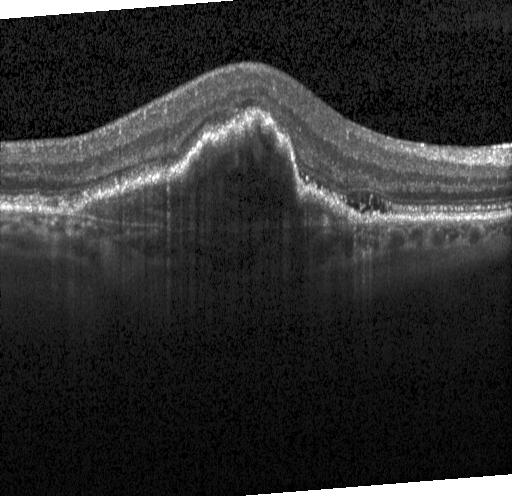

Retinal OCT cross-section
Impression: a choroidal neovascular membrane.